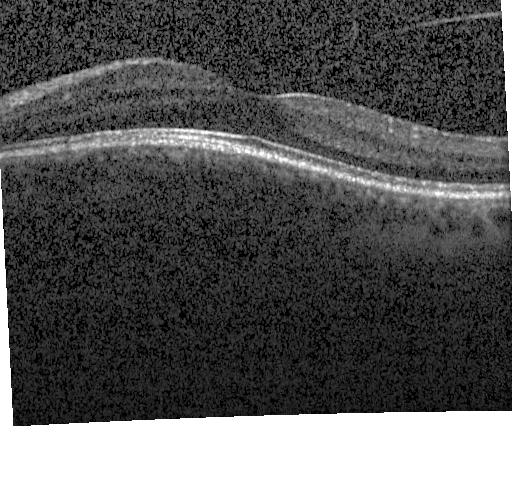
Neither choroidal neovascularization, diabetic macular edema, nor drusen.